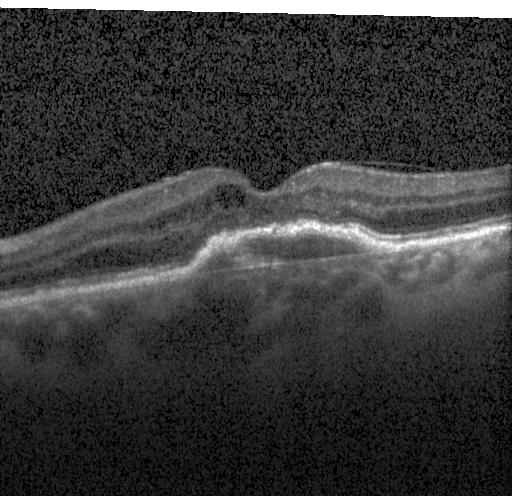 Diagnosis: CNV.